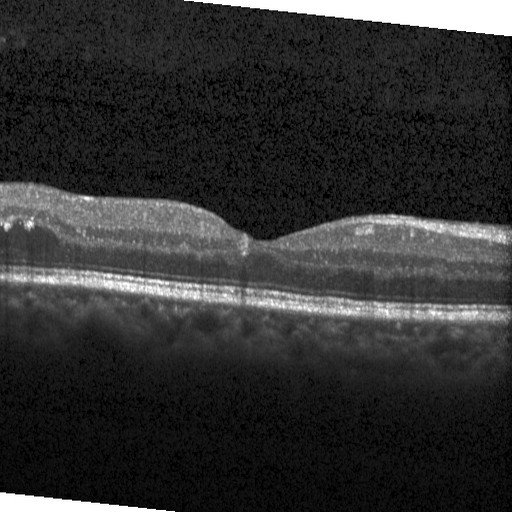 Optical coherence tomography B-scan — Impression: diabetic macular edema.